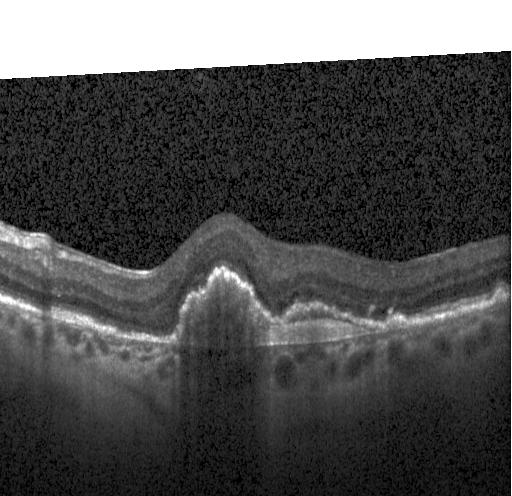
Impression: a choroidal neovascular membrane.